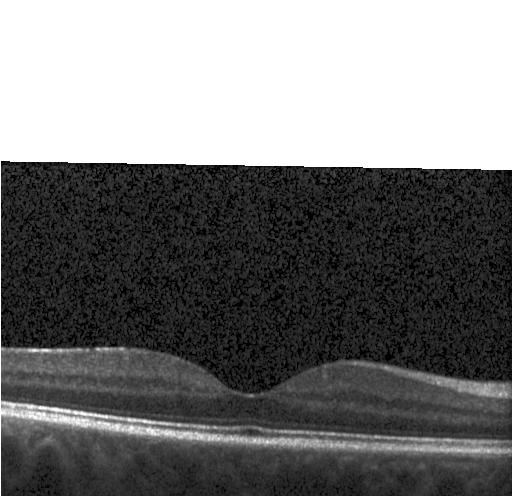

Spectral-domain OCT, optical coherence tomography B-scan — Impression: no choroidal neovascularization, diabetic macular edema, or drusen.